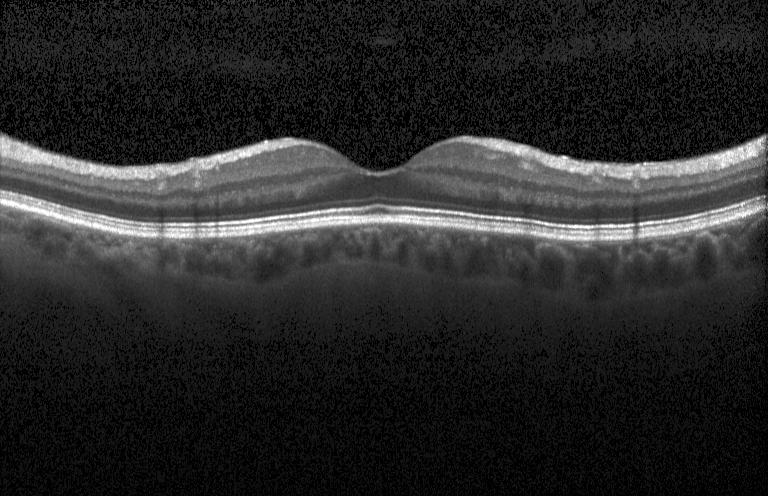
Impression: no choroidal neovascularization, diabetic macular edema, or drusen.